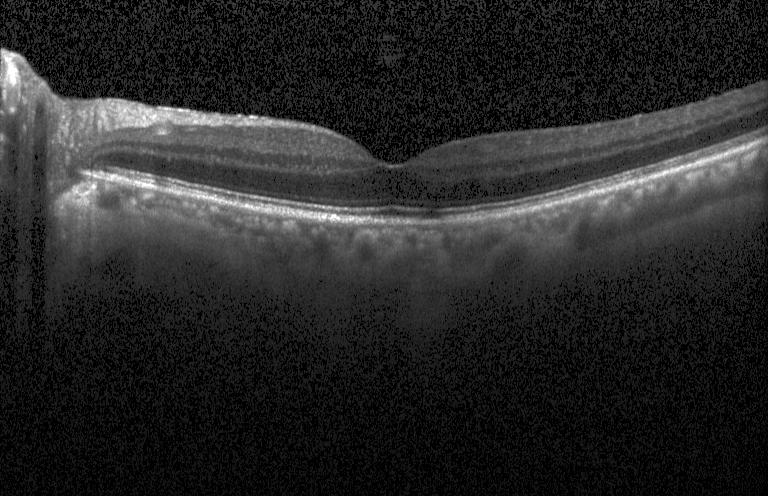 Dx: neither CNV, DME, nor drusen.